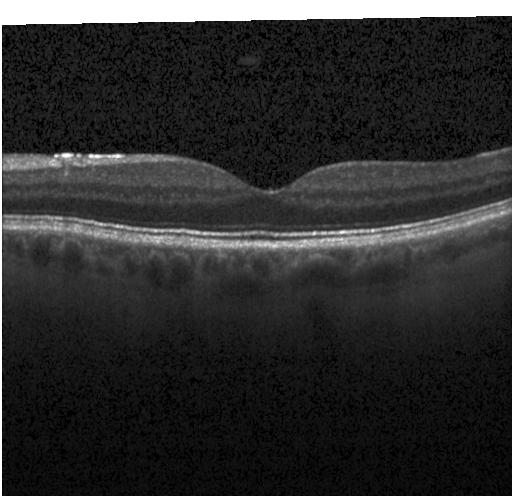 Optical coherence tomography B-scan, Heidelberg Spectralis OCT system, fovea-centered, spectral-domain OCT.
Dx: no evidence of choroidal neovascularization, diabetic macular edema, or drusen.